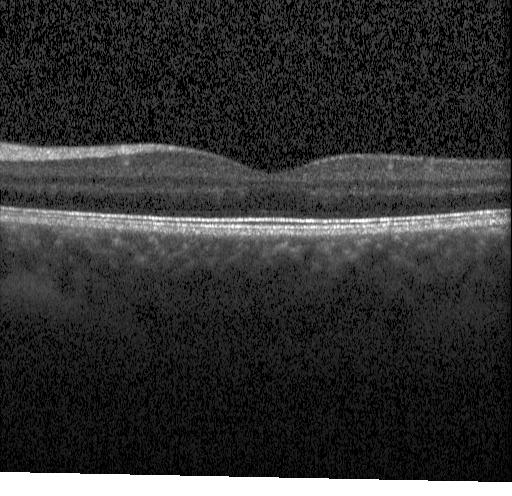
Optical coherence tomography B-scan · spectral-domain optical coherence tomography · instrument: Heidelberg Spectralis. Impression: no choroidal neovascularization, no diabetic macular edema, and no drusen.